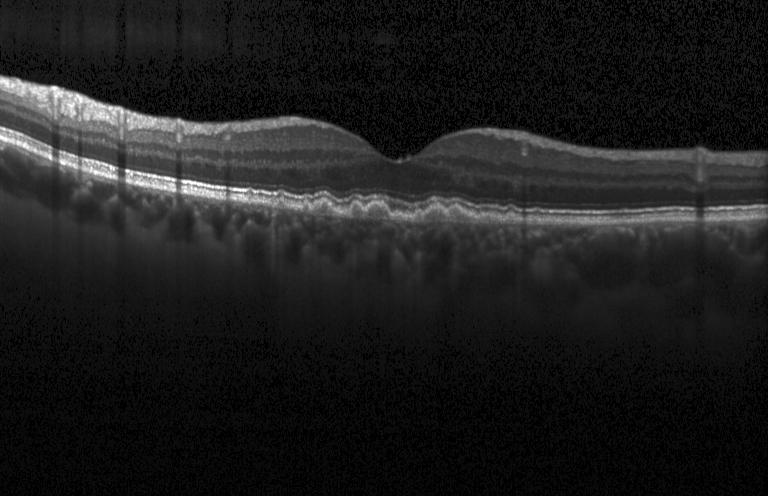 Retinal OCT cross-section; Heidelberg Spectralis; spectral-domain OCT; fovea-centered
Diagnosis: multiple drusen.